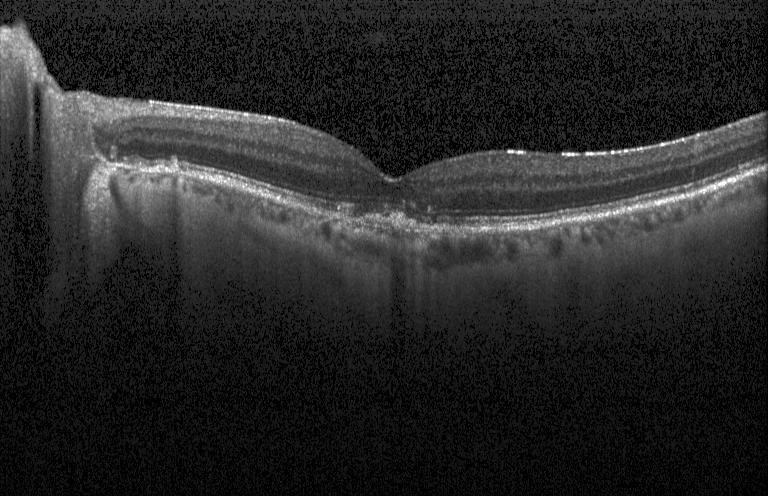 Finding: choroidal neovascularization (CNV).